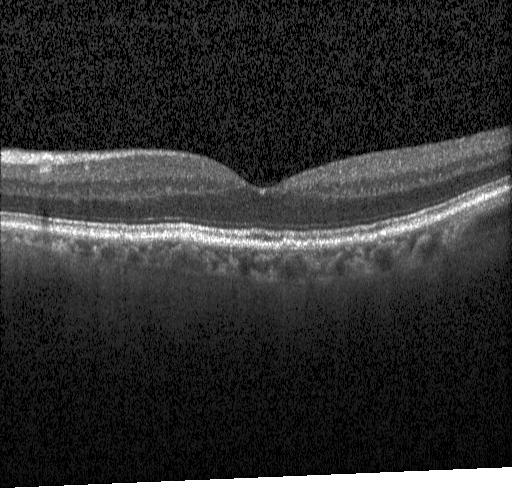

Retinal OCT cross-section. Dx: no evidence of choroidal neovascularization, diabetic macular edema, or drusen.